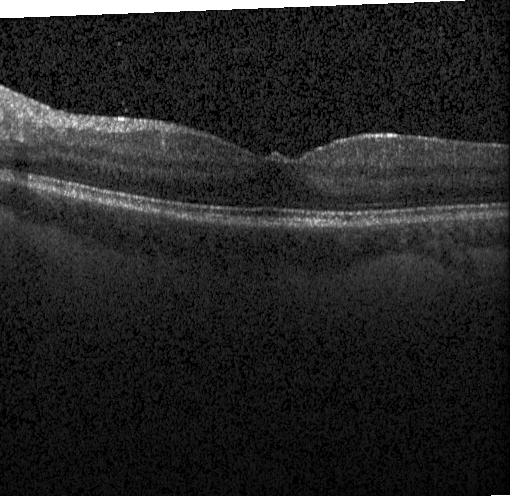
Acquired on a Heidelberg Spectralis; optical coherence tomography B-scan; spectral-domain OCT; centered on the fovea.
No evidence of CNV, DME, or drusen.